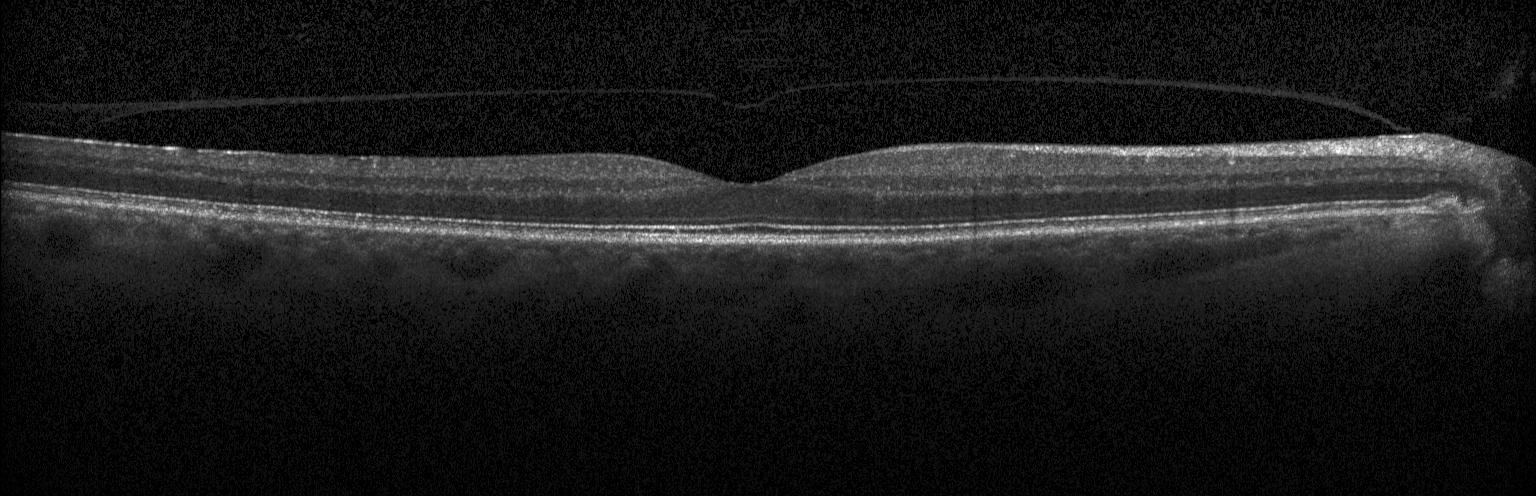
Macular OCT: no CNV, DME, or drusen.